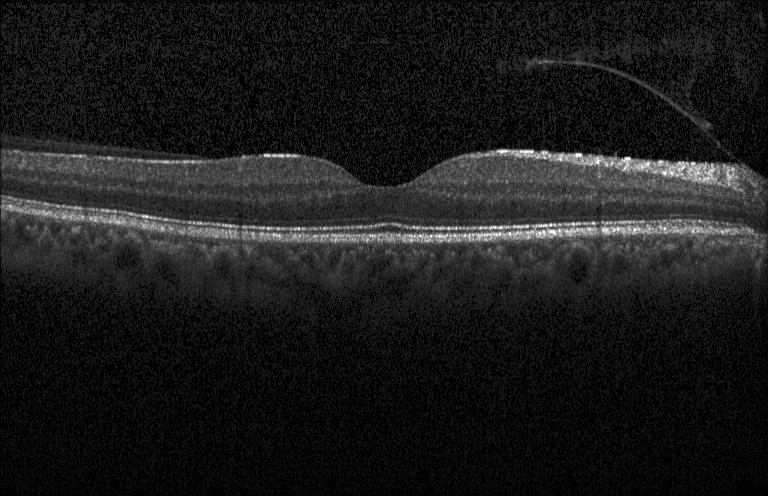

Spectral-domain optical coherence tomography. Centered on the fovea. Acquired on a Heidelberg Spectralis. OCT line scan. Finding: neither CNV, DME, nor drusen.